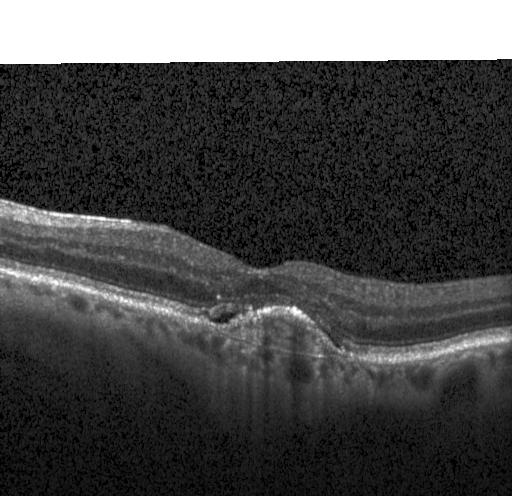

Spectral-domain optical coherence tomography. Fovea-centered. Heidelberg Spectralis. OCT line scan. Diagnosis: choroidal neovascularization (CNV).